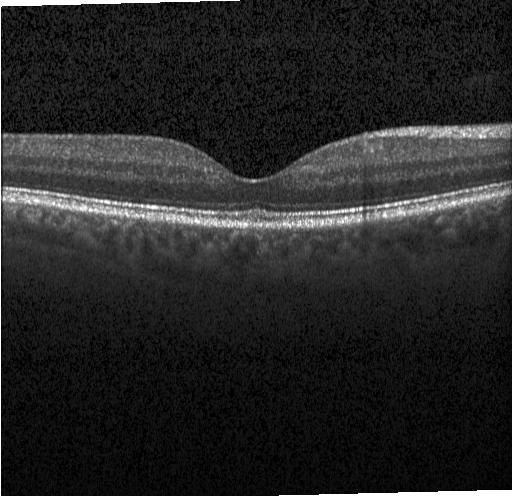
OCT finding: neither choroidal neovascularization, diabetic macular edema, nor drusen.